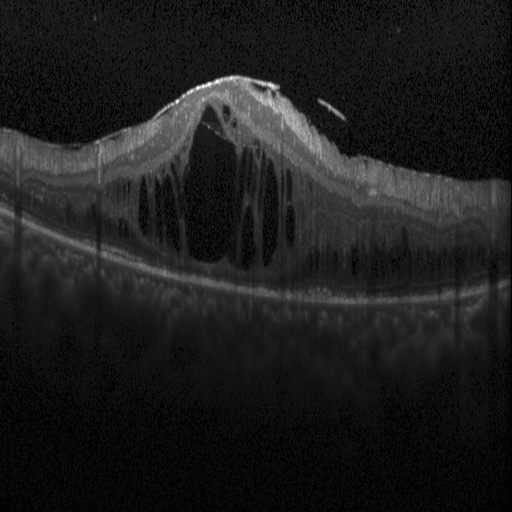 Macular OCT demonstrating diabetic macular edema.